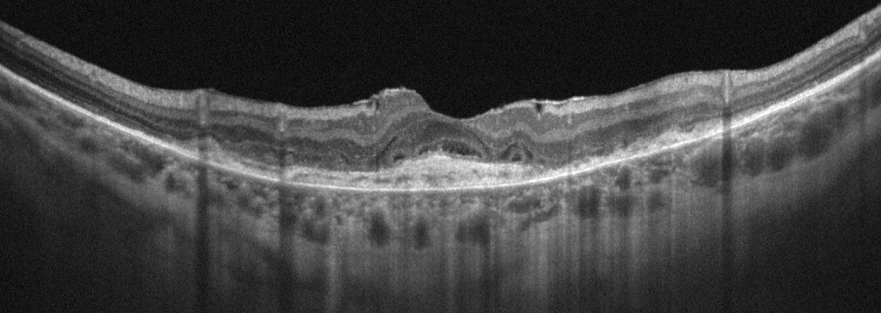 Optical coherence tomography scan
Finding: AMD.